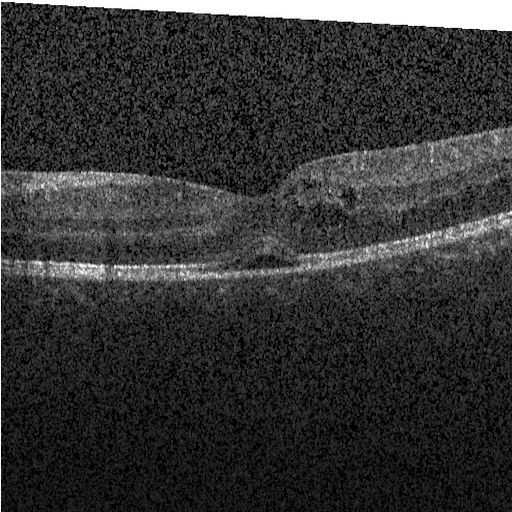
Spectral-domain OCT, acquired on a Heidelberg Spectralis, OCT line scan — Macular OCT: diabetic macular edema.